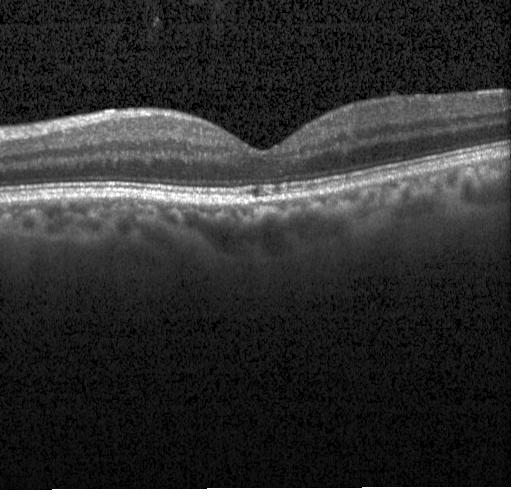

SD-OCT. Through the macula. Instrument: Heidelberg Spectralis. Optical coherence tomography B-scan — Dx: no evidence of CNV, DME, or drusen.